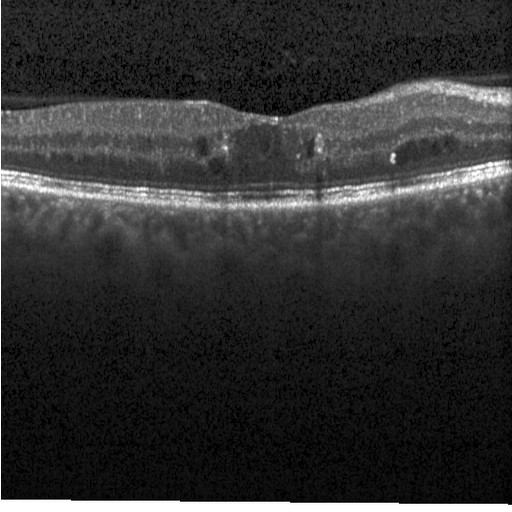
Optical coherence tomography B-scan, horizontal scan through the fovea, Heidelberg Spectralis — Diagnosis: diabetic macular edema (DME).